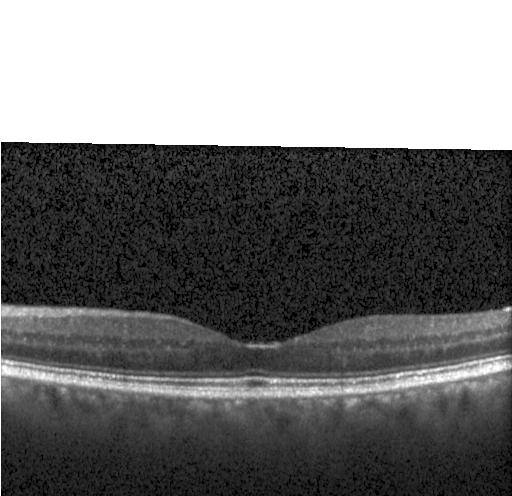

Retinal OCT B-scan. Impression: neither choroidal neovascularization, diabetic macular edema, nor drusen.